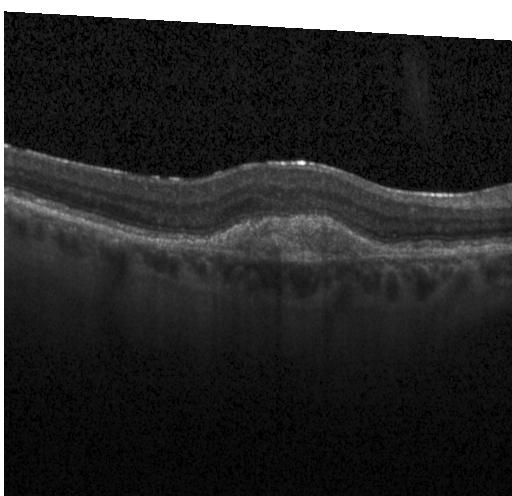 OCT finding: choroidal neovascularization.